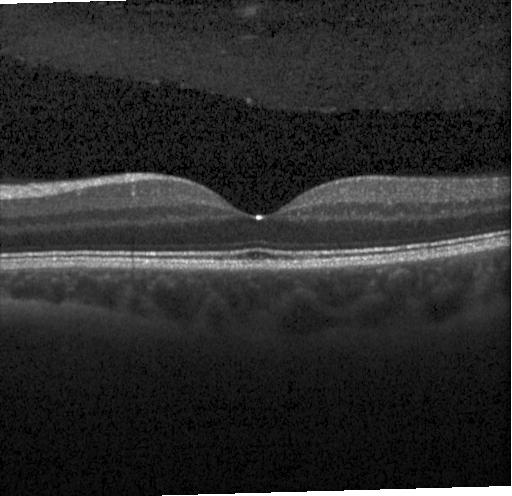 Dx: neither choroidal neovascularization, diabetic macular edema, nor drusen.